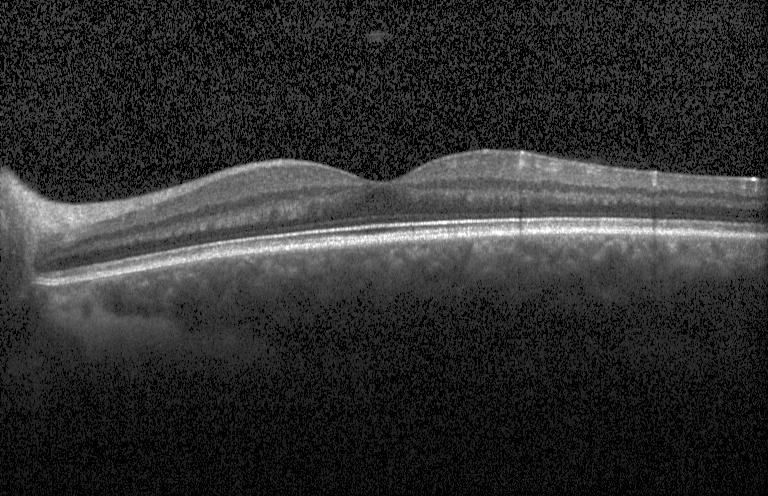
Finding: no choroidal neovascularization, diabetic macular edema, or drusen.